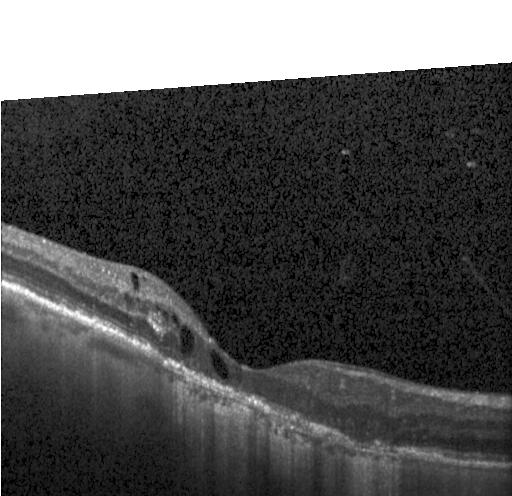 Fovea-centered · optical coherence tomography B-scan · acquired on a Heidelberg Spectralis · spectral-domain optical coherence tomography. Macular OCT: a choroidal neovascular membrane.